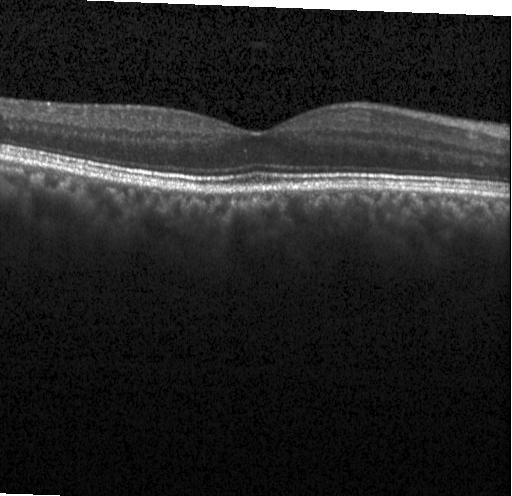

Retinal OCT cross-section — This B-scan demonstrates no choroidal neovascularization, diabetic macular edema, or drusen.